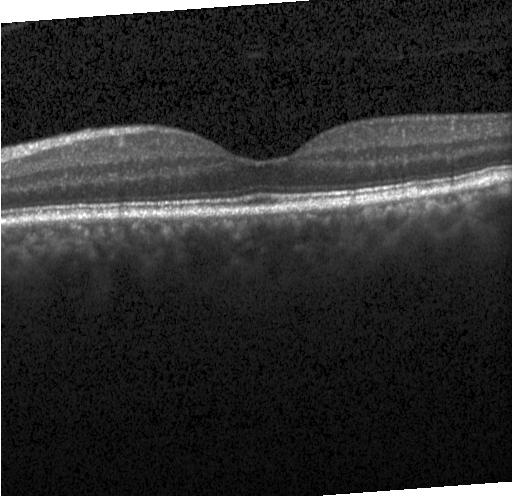

Macular OCT: neither choroidal neovascularization, diabetic macular edema, nor drusen.